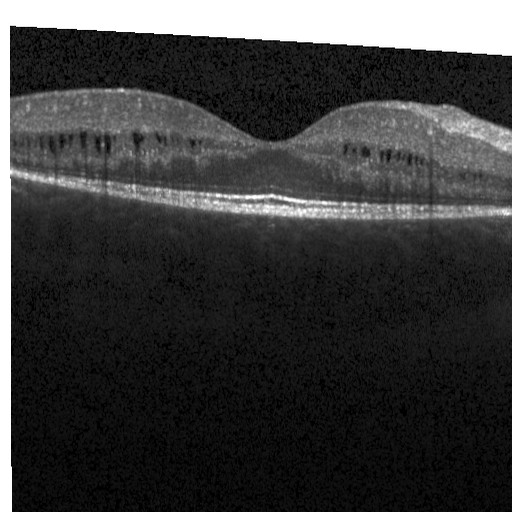
Diabetic macular edema (DME).